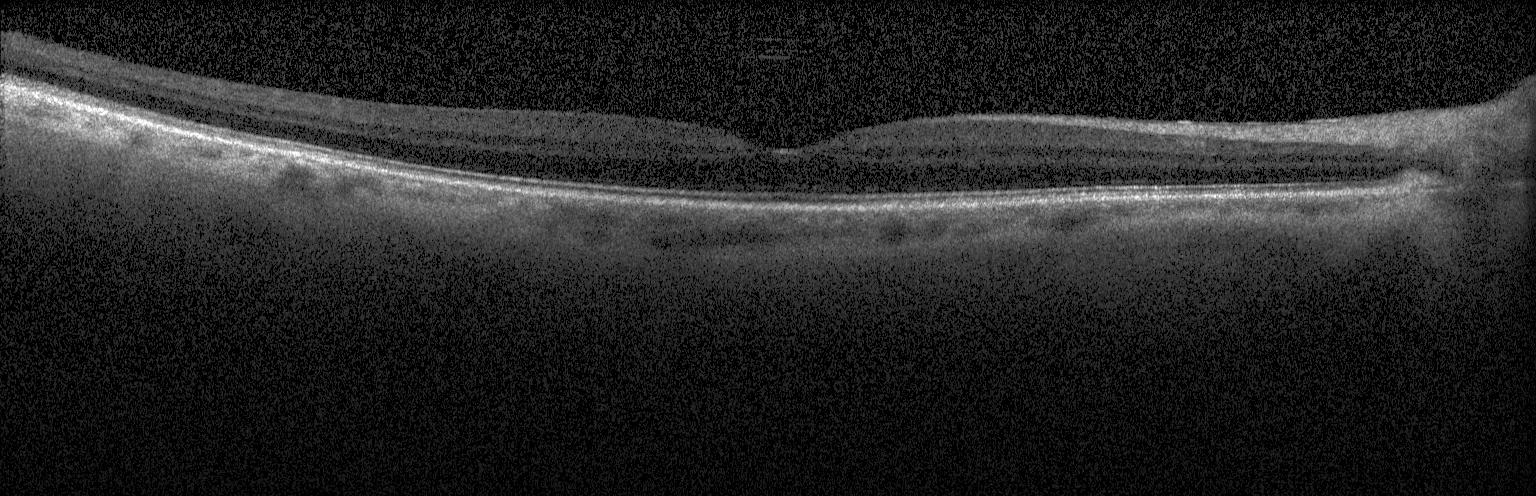 Instrument: Heidelberg Spectralis · SD-OCT · OCT line scan. Diagnosis: no evidence of CNV, DME, or drusen.